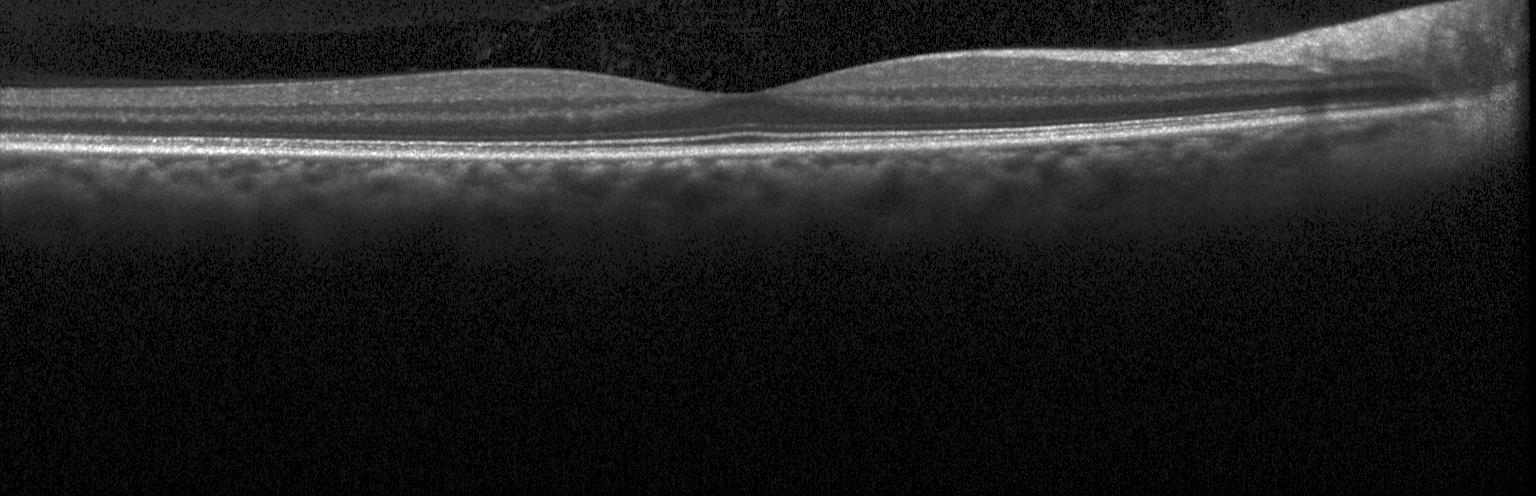 OCT B-scan — This B-scan demonstrates no choroidal neovascularization, no diabetic macular edema, and no drusen.